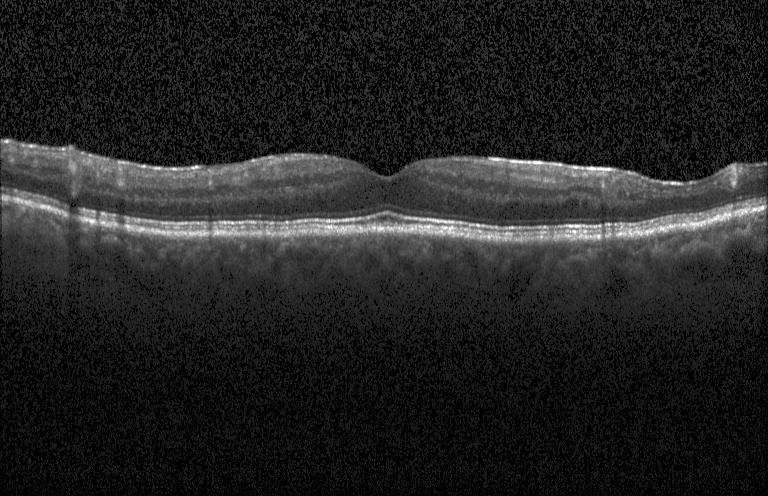
OCT scan showing no choroidal neovascularization, no diabetic macular edema, and no drusen.